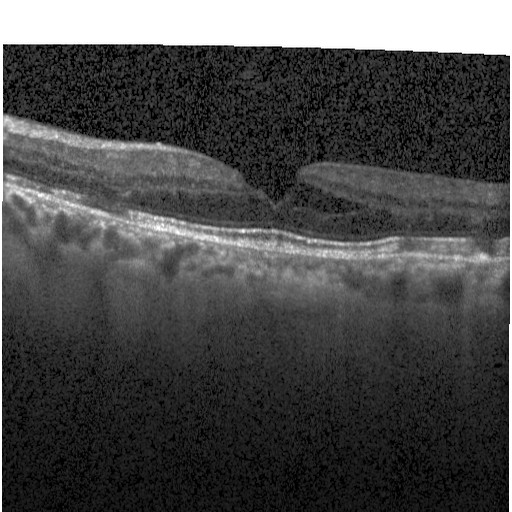

Centered on the fovea, optical coherence tomography B-scan
Diagnosis: DME.